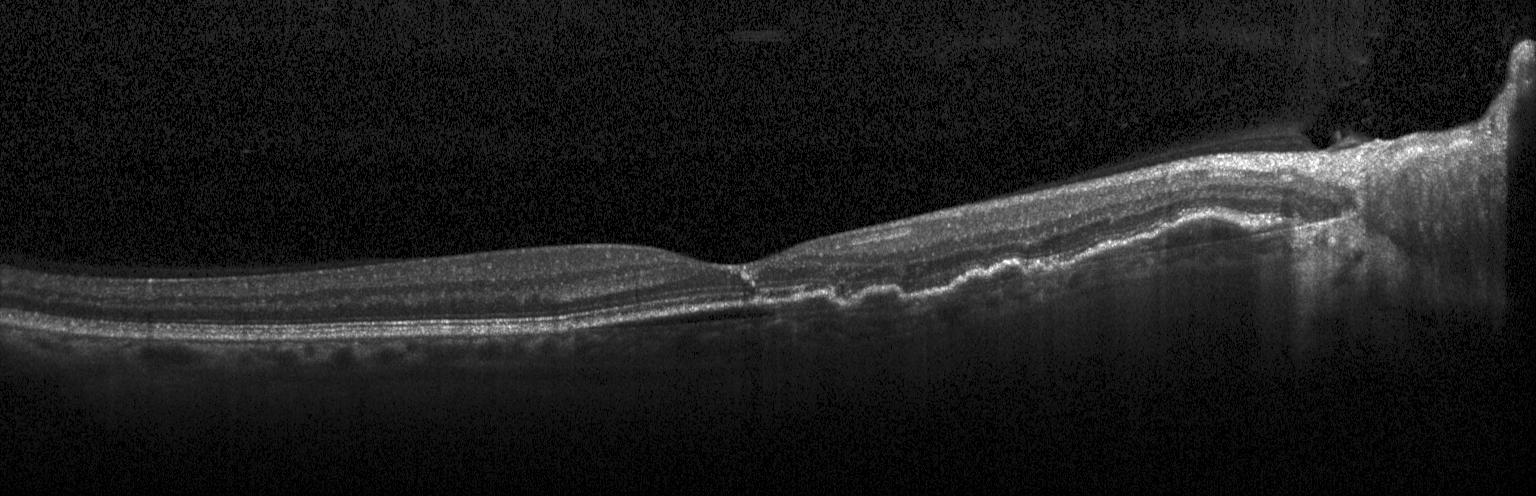 OCT line scan · spectral-domain optical coherence tomography · fovea-centered · acquired on a Heidelberg Spectralis. Diagnosis: a choroidal neovascular membrane.